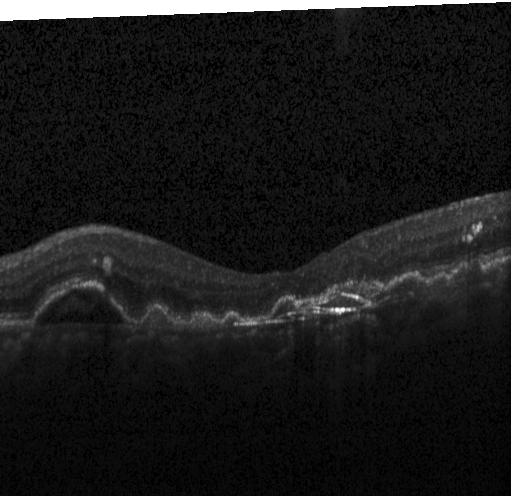
Finding: choroidal neovascularization (CNV).